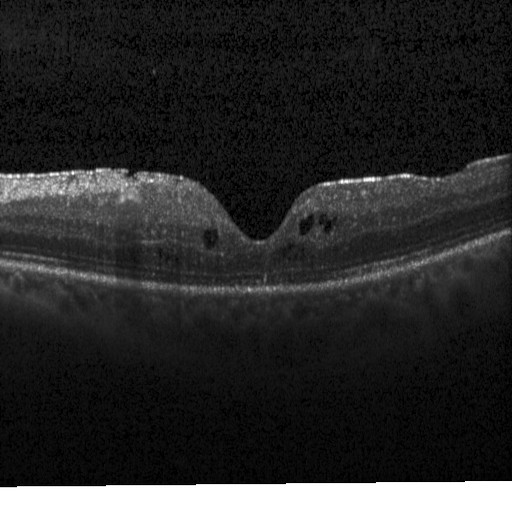 Optical coherence tomography B-scan — Finding: diabetic macular edema (DME).